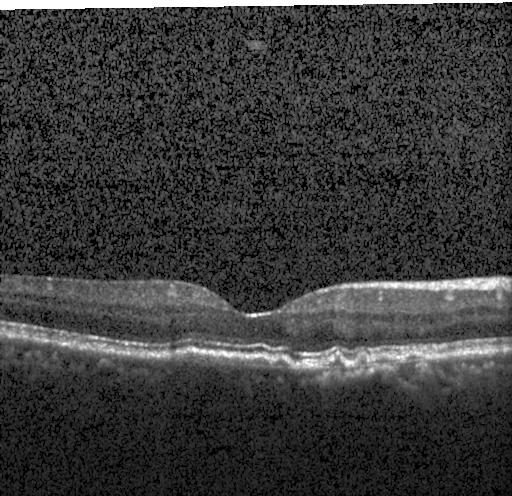

Instrument: Heidelberg Spectralis · OCT line scan · centered on the fovea
Finding: sub-RPE drusenoid deposits.